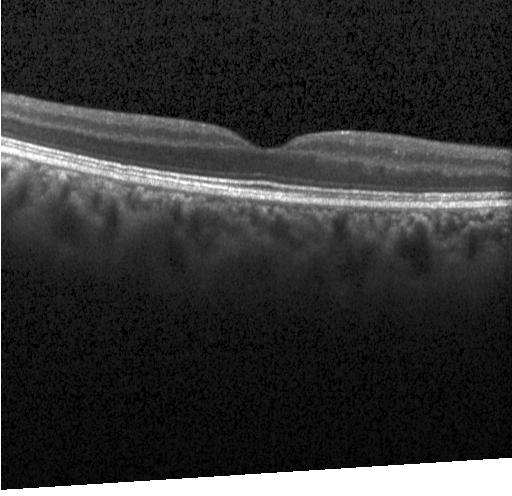

Spectral-domain optical coherence tomography. Optical coherence tomography B-scan. OCT finding: no choroidal neovascularization, diabetic macular edema, or drusen.